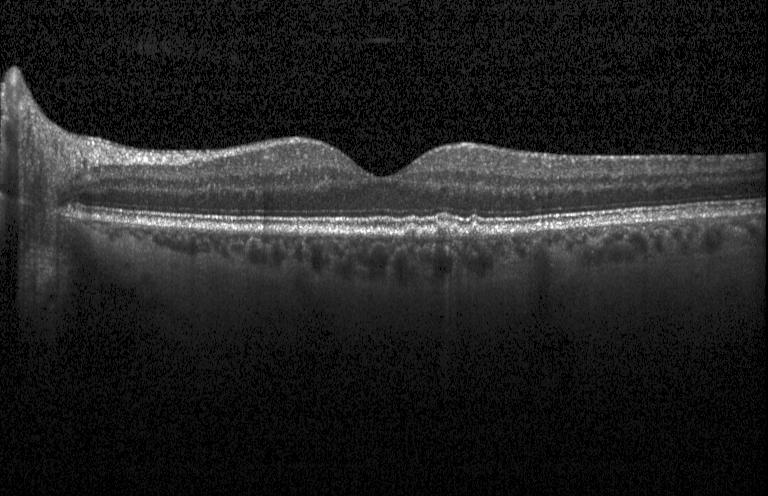
SD-OCT; retinal OCT cross-section; Heidelberg Spectralis; fovea-centered. Dx: drusen.